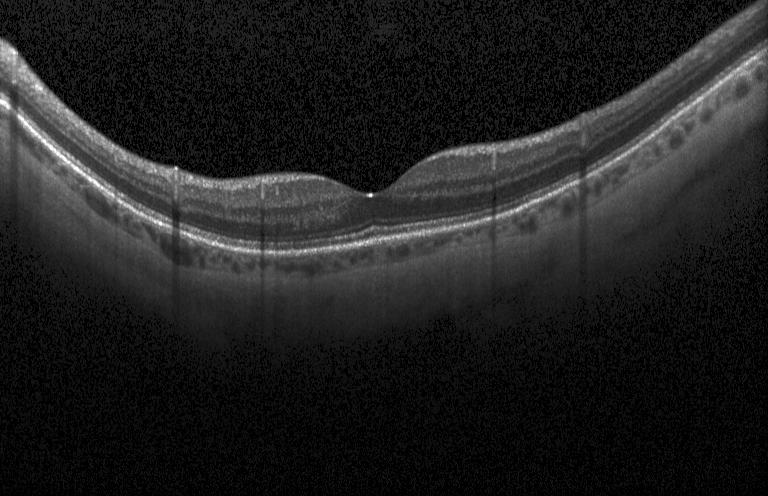 Acquired on a Heidelberg Spectralis · optical coherence tomography B-scan · SD-OCT — Diagnosis: neither choroidal neovascularization, diabetic macular edema, nor drusen.